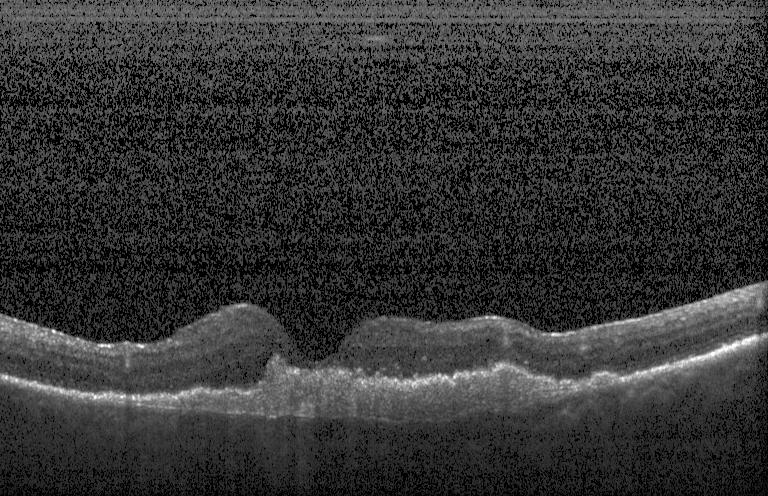
Retinal OCT cross-section. Centered on the fovea. Spectral-domain OCT. Heidelberg Spectralis OCT system. Finding: a choroidal neovascular membrane.